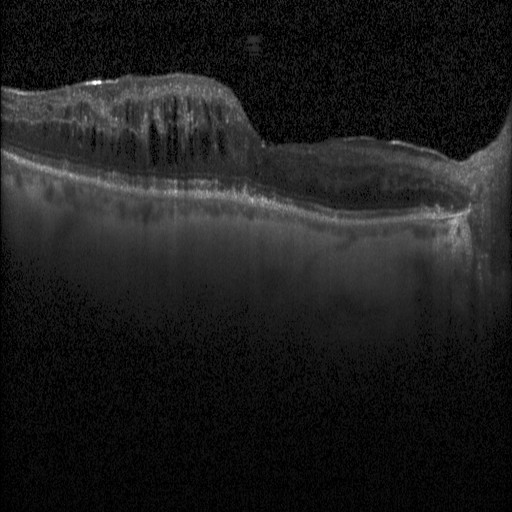
Macular OCT: diabetic macular edema.